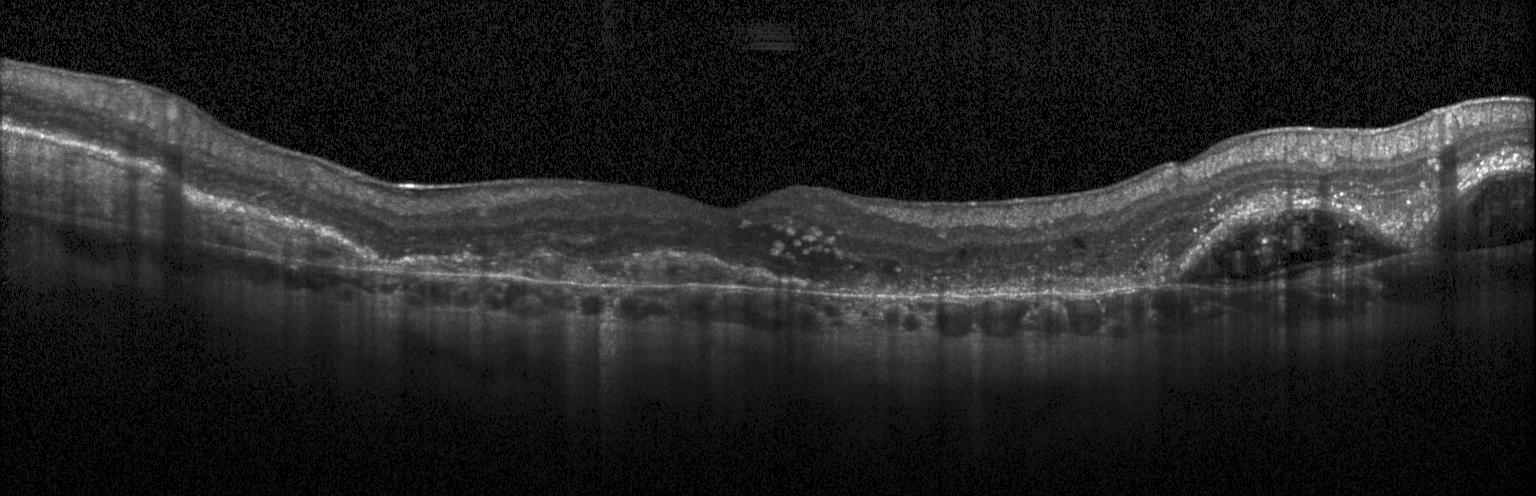

CNV.